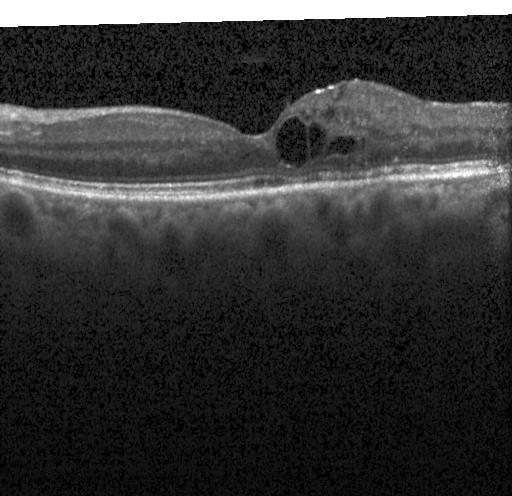
OCT finding: diabetic macular edema (DME).